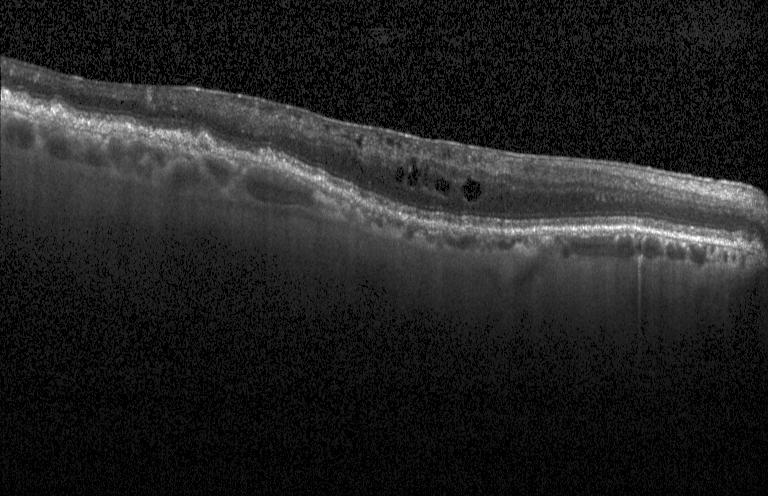
Spectral-domain OCT. Retinal OCT cross-section
Assessment: CNV.